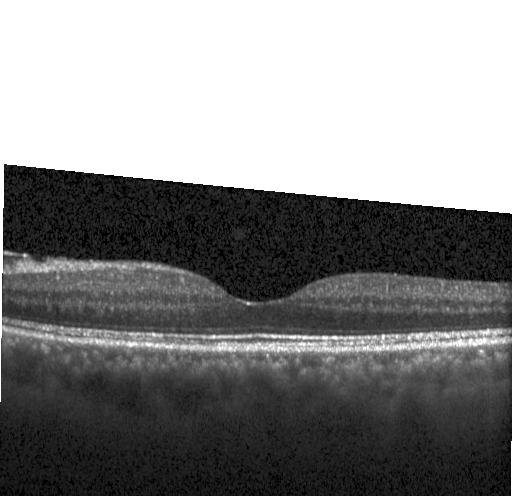

Heidelberg Spectralis. Retinal OCT cross-section.
This B-scan demonstrates no evidence of choroidal neovascularization, diabetic macular edema, or drusen.